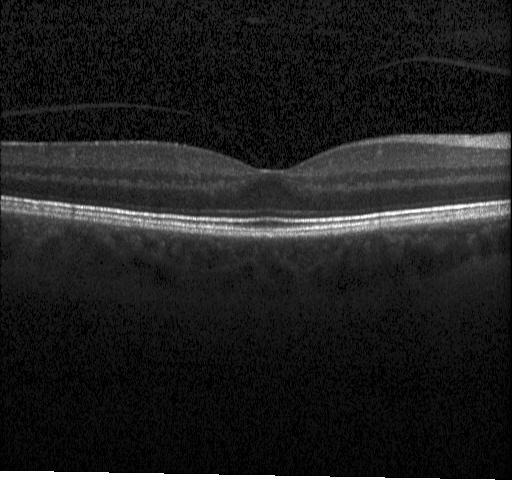 Impression: no choroidal neovascularization, no diabetic macular edema, and no drusen.